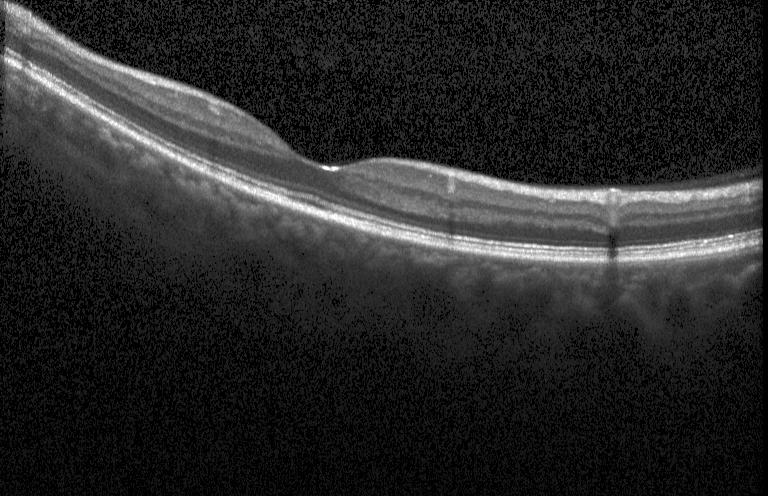 Optical coherence tomography B-scan · macular scan · spectral-domain optical coherence tomography · Heidelberg Spectralis.
The scan shows neither CNV, DME, nor drusen.